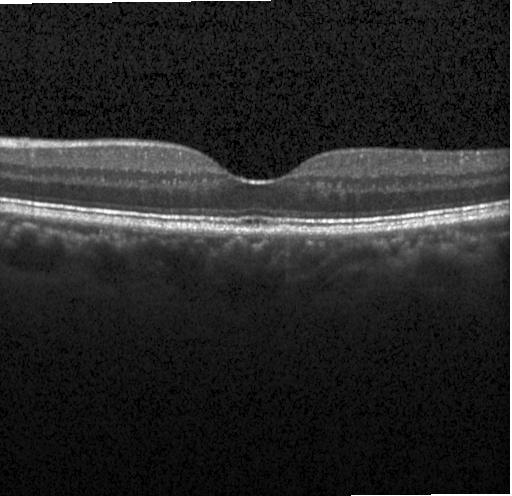

Assessment: no evidence of choroidal neovascularization, diabetic macular edema, or drusen.